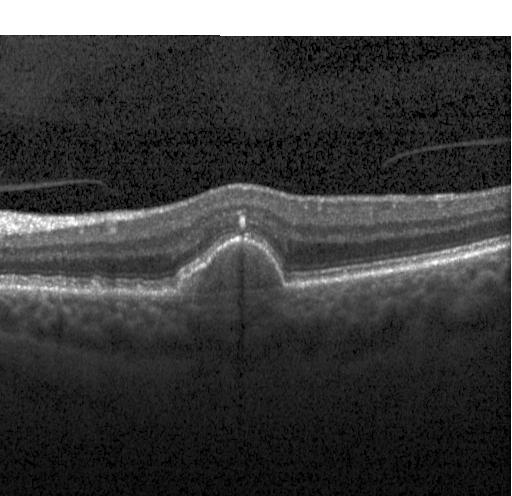 Retinal OCT cross-section. Impression: a choroidal neovascular membrane.